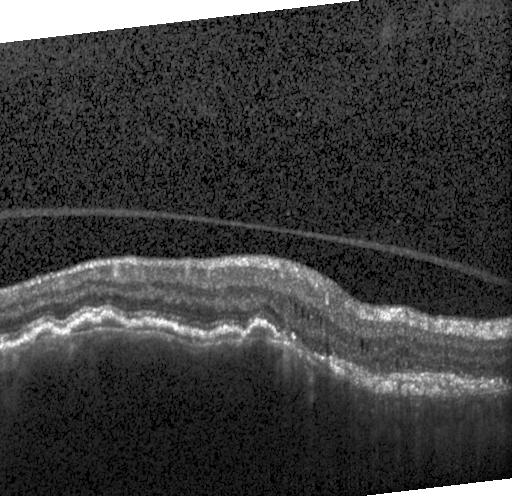 Macular scan · spectral-domain OCT · OCT line scan · acquired on a Heidelberg Spectralis.
Impression: CNV.